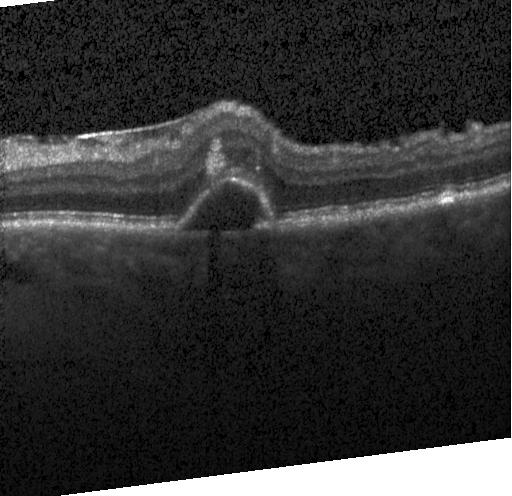

Heidelberg Spectralis OCT system. SD-OCT. OCT line scan
Dx: a choroidal neovascular membrane.